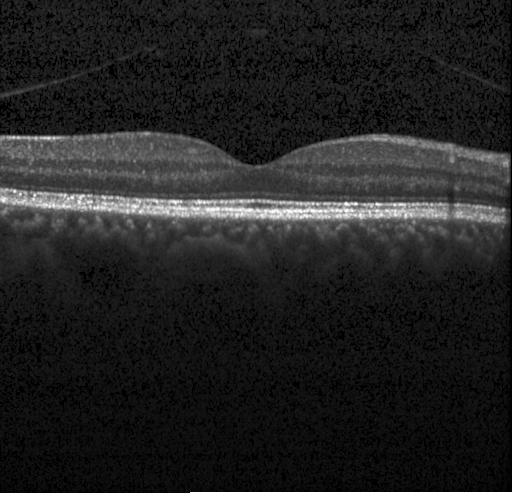 Centered on the fovea; OCT line scan.
Dx: no evidence of CNV, DME, or drusen.